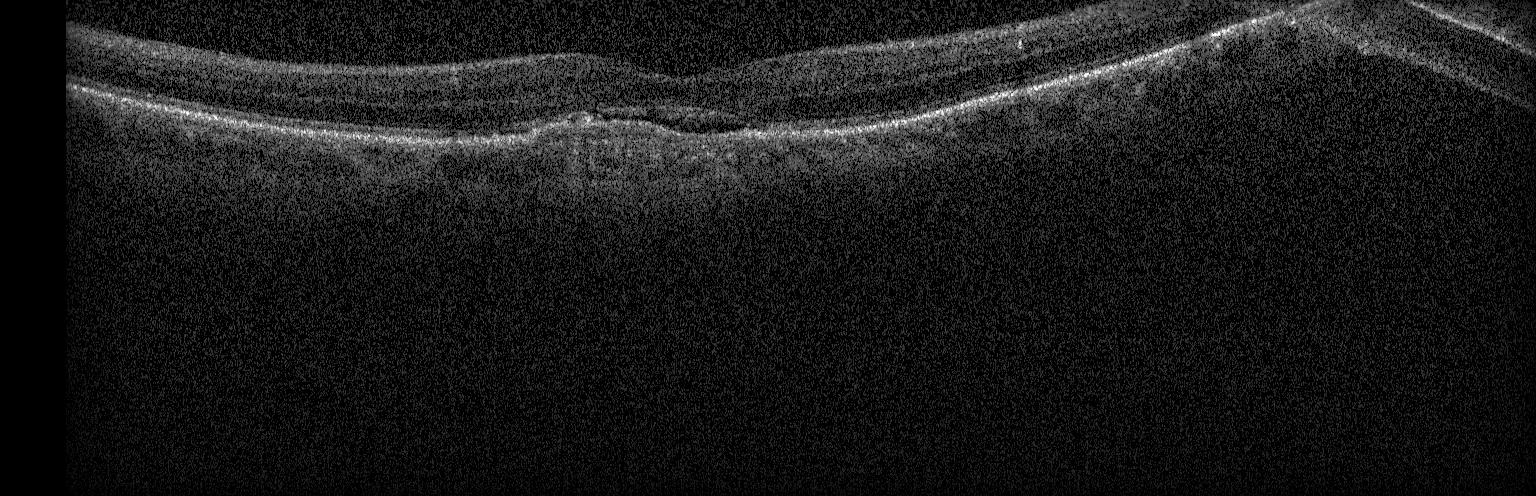

Spectral-domain OCT B-scan: a choroidal neovascular membrane.